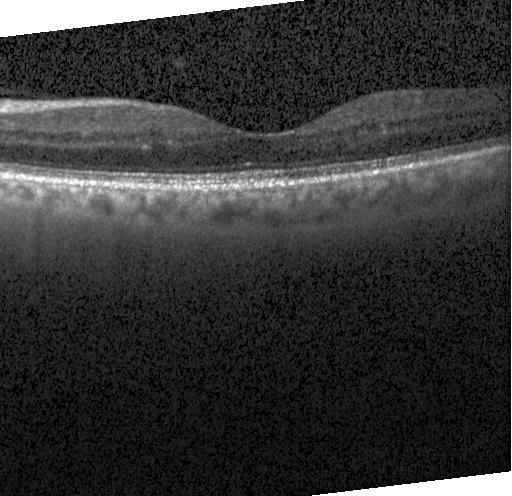
Finding: no choroidal neovascularization, diabetic macular edema, or drusen.